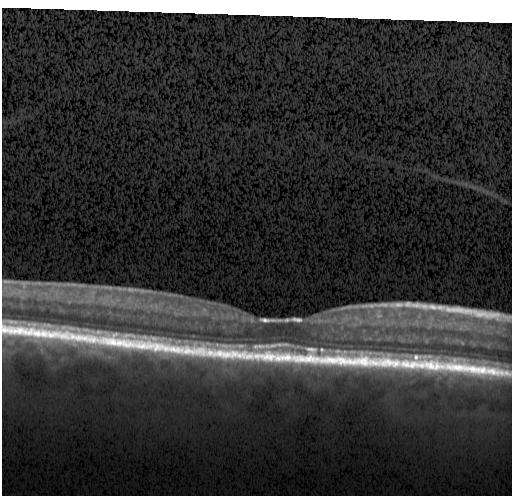 OCT B-scan showing neither choroidal neovascularization, diabetic macular edema, nor drusen.